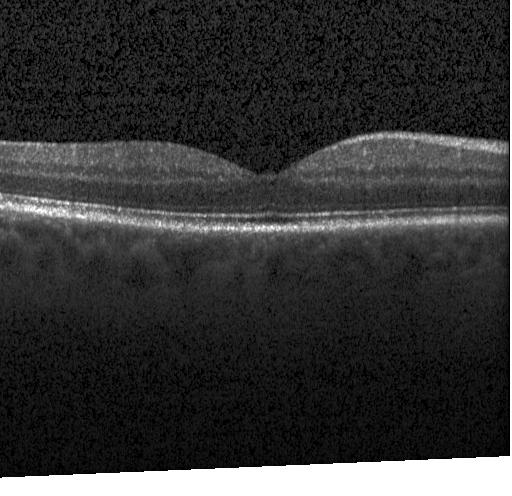
Impression: no choroidal neovascularization, diabetic macular edema, or drusen.